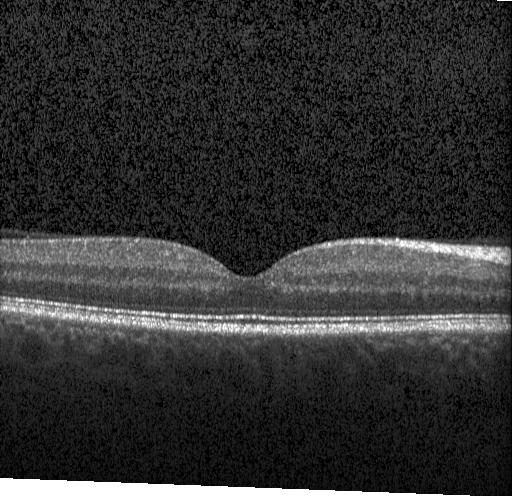 Retinal OCT cross-section. Heidelberg Spectralis. Centered on the fovea
This B-scan demonstrates no choroidal neovascularization, diabetic macular edema, or drusen.